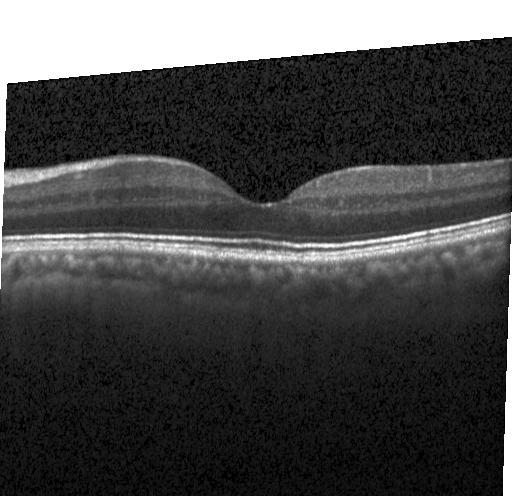
OCT finding: no choroidal neovascularization, diabetic macular edema, or drusen.